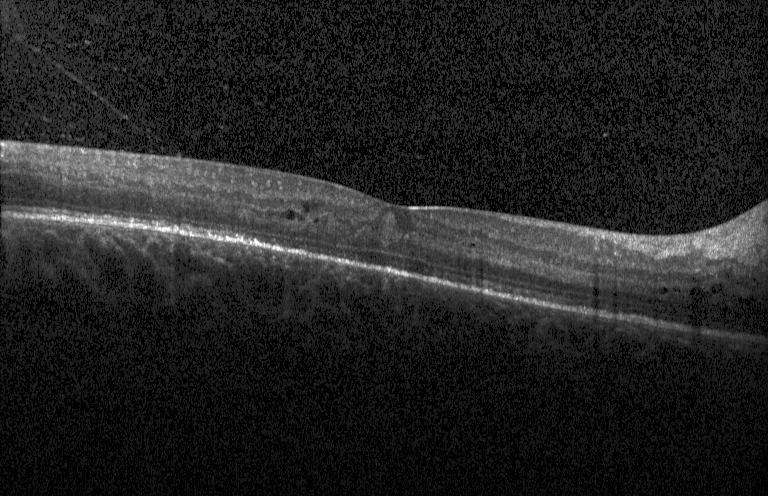
Diagnosis: diabetic macular edema (DME).